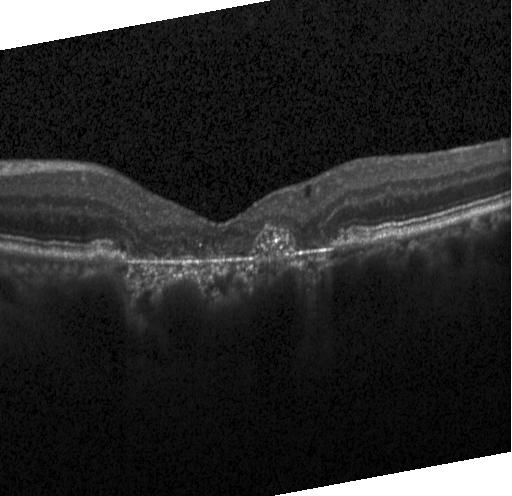
Retinal OCT cross-section.
OCT finding: a choroidal neovascular membrane.